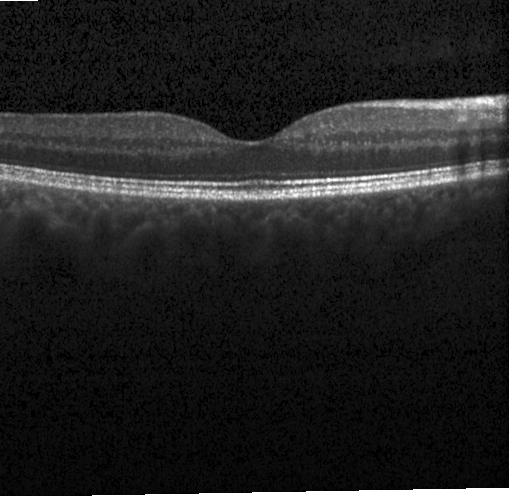
Dx: no evidence of choroidal neovascularization, diabetic macular edema, or drusen.